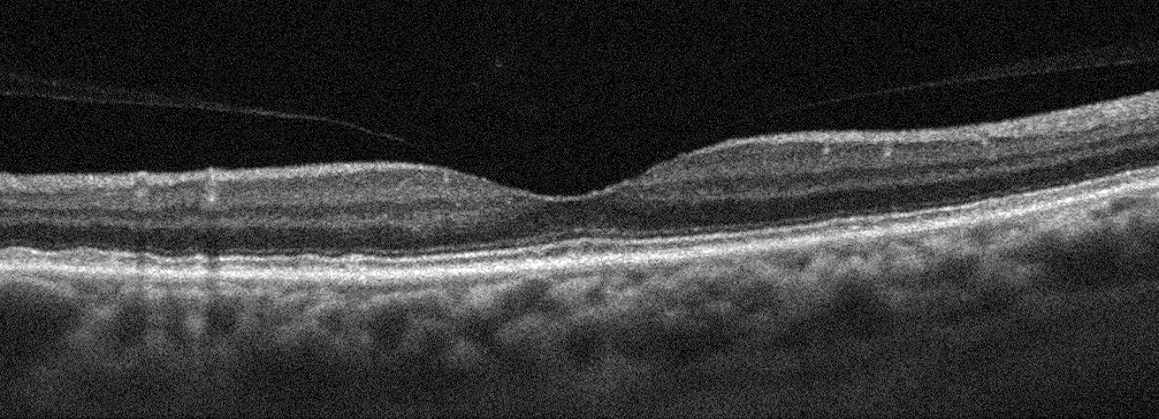
Oculus sinister, through the macula, OCT B-scan.
This B-scan demonstrates age-related macular degeneration (AMD).